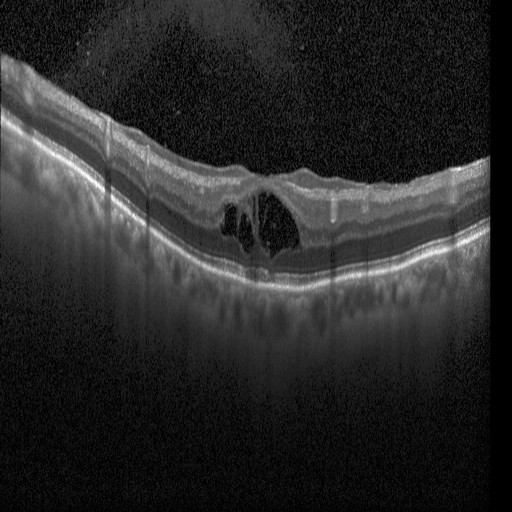

Horizontal scan through the fovea · instrument: Heidelberg Spectralis · retinal OCT B-scan · SD-OCT.
Impression: diabetic macular edema.